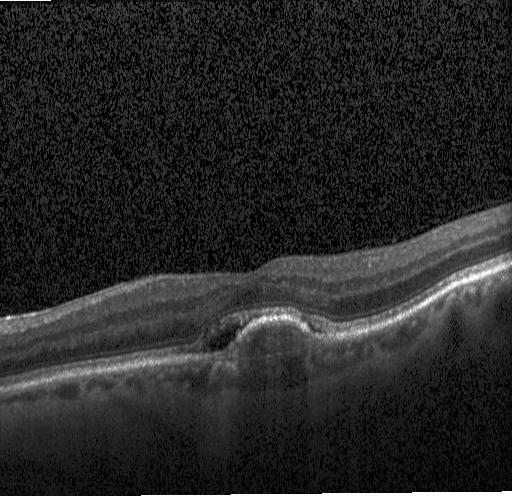 OCT B-scan.
The scan shows a choroidal neovascular membrane.